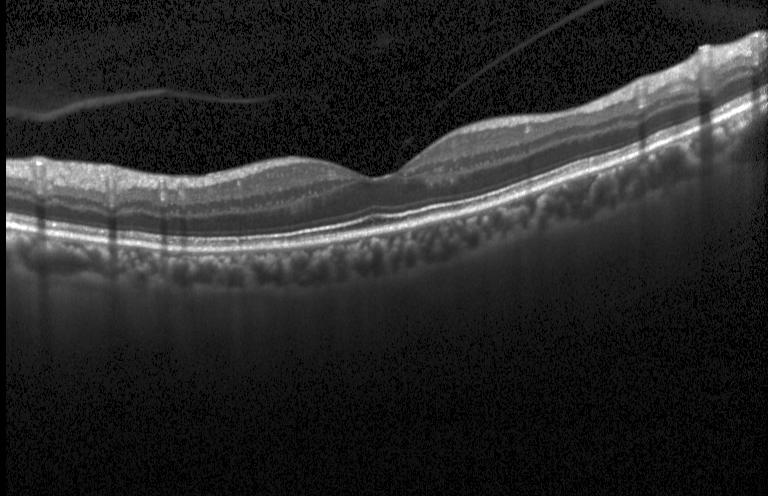 Diagnosis: neither choroidal neovascularization, diabetic macular edema, nor drusen.